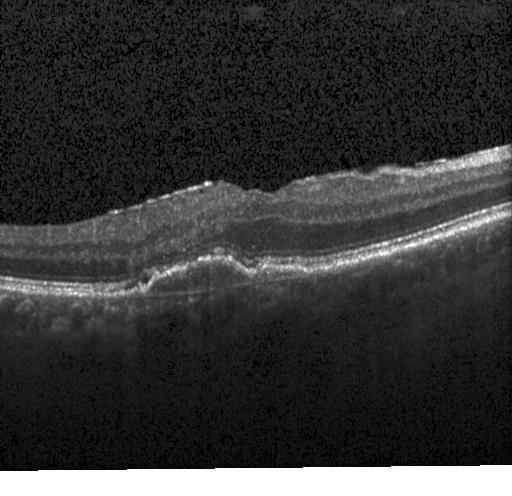 Retinal OCT B-scan. Acquired on a Heidelberg Spectralis. Horizontal scan through the fovea
Finding: choroidal neovascularization (CNV).